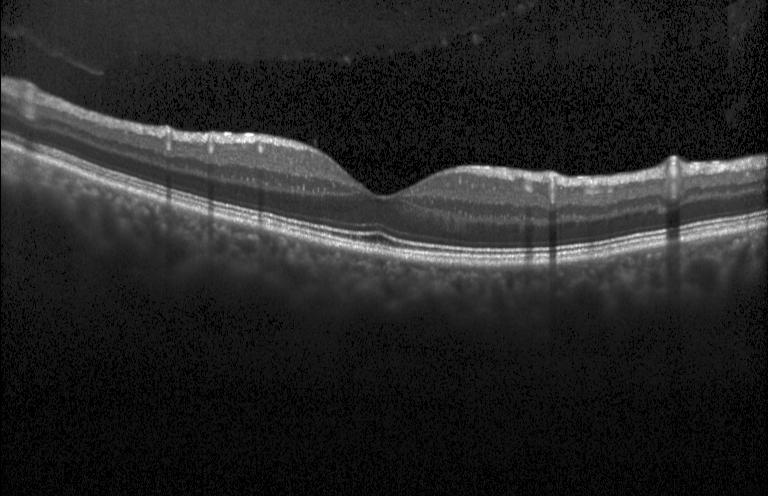
OCT line scan, spectral-domain optical coherence tomography — OCT finding: neither CNV, DME, nor drusen.